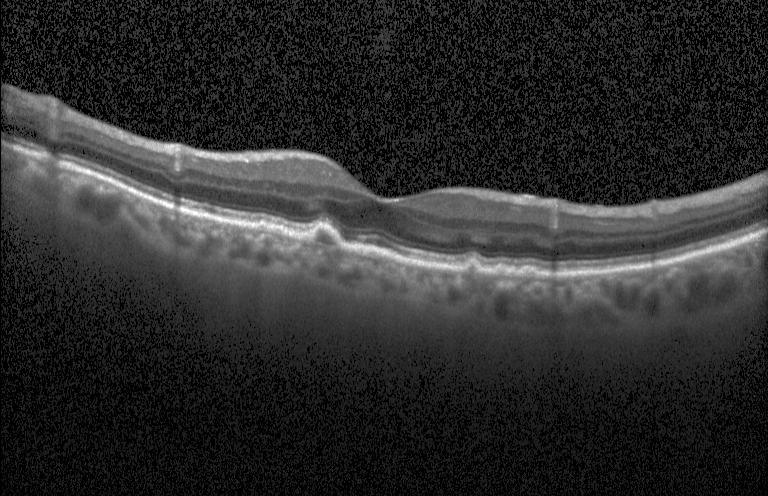 Spectral-domain OCT B-scan: sub-RPE drusenoid deposits.